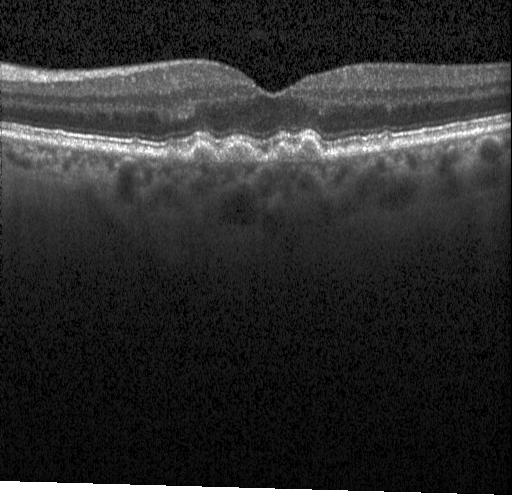 Dx: sub-RPE drusenoid deposits.